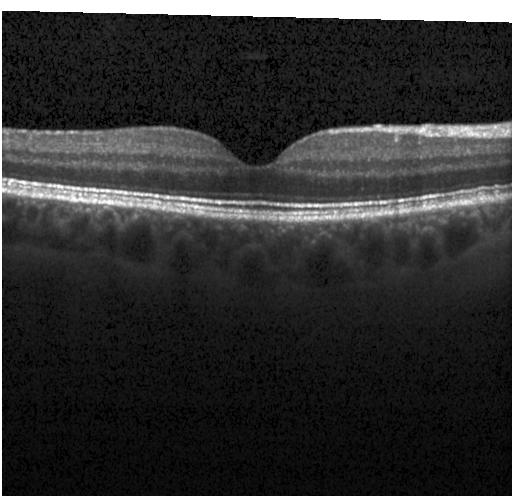
OCT B-scan — Assessment: no choroidal neovascularization, diabetic macular edema, or drusen.